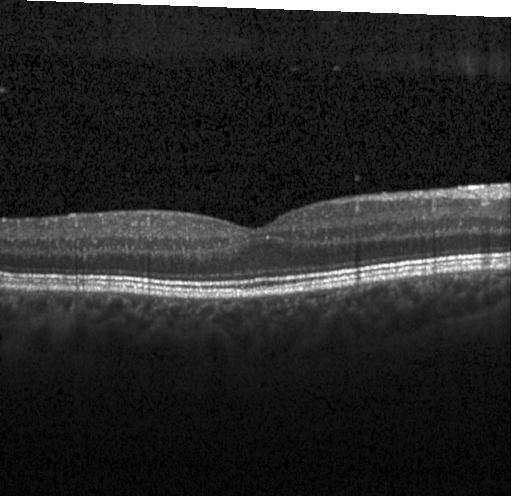 Impression: neither choroidal neovascularization, diabetic macular edema, nor drusen.